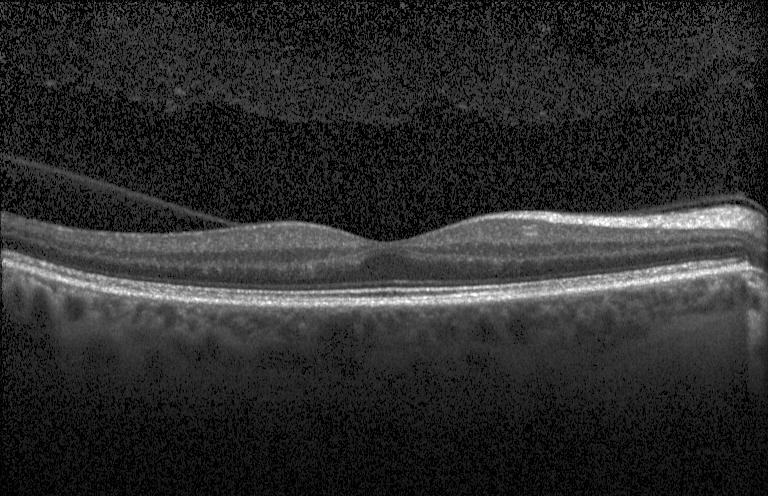
Spectral-domain optical coherence tomography. OCT line scan. Fovea-centered. This B-scan demonstrates no evidence of CNV, DME, or drusen.